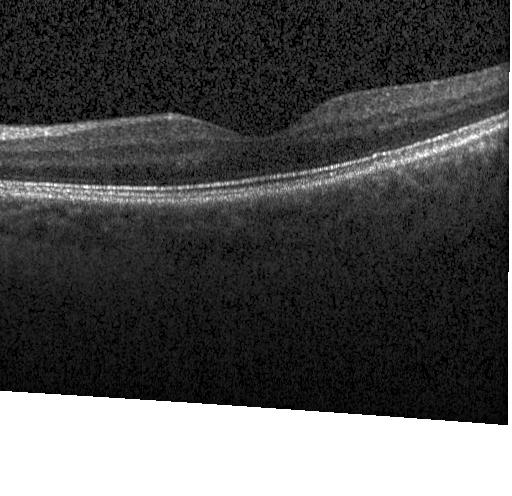 Optical coherence tomography scan.
Diagnosis: neither choroidal neovascularization, diabetic macular edema, nor drusen.